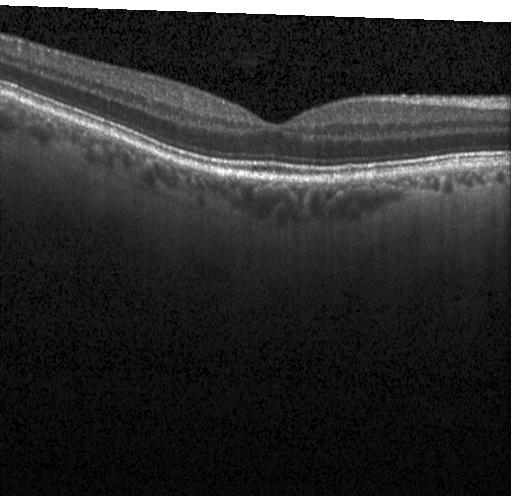 Optical coherence tomography scan · spectral-domain optical coherence tomography · macular scan · Heidelberg Spectralis. No evidence of choroidal neovascularization, diabetic macular edema, or drusen.